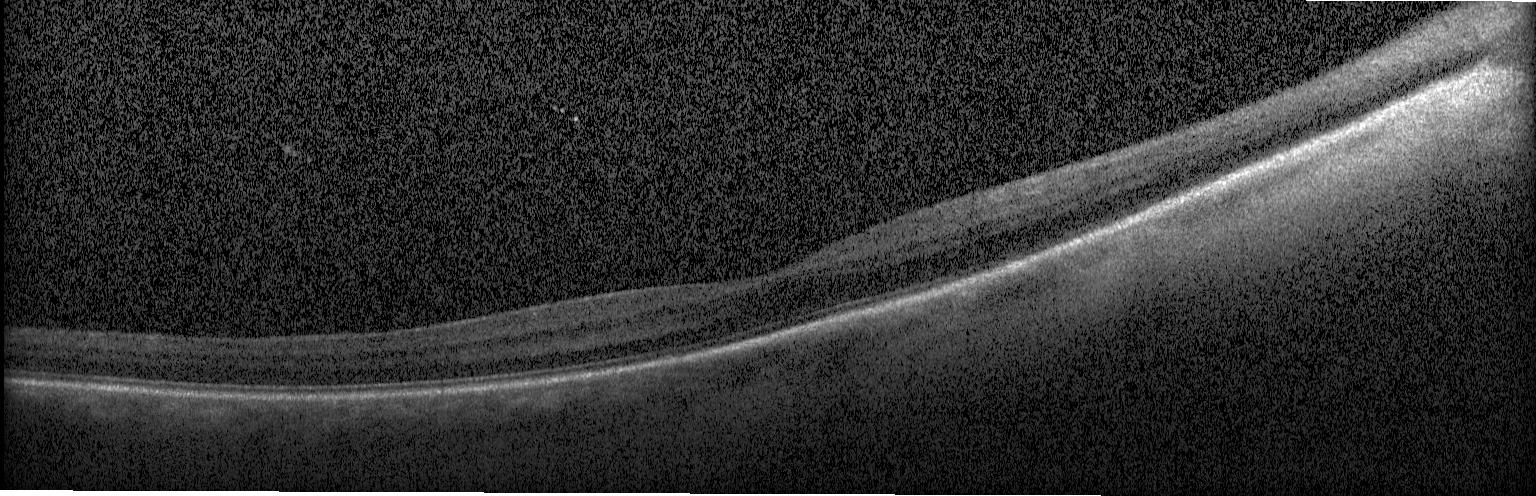 Optical coherence tomography B-scan; instrument: Heidelberg Spectralis; SD-OCT; fovea-centered
The scan shows no choroidal neovascularization, diabetic macular edema, or drusen.